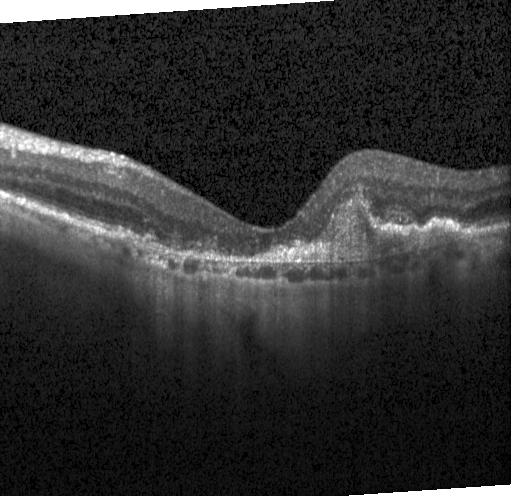
The scan shows choroidal neovascularization.